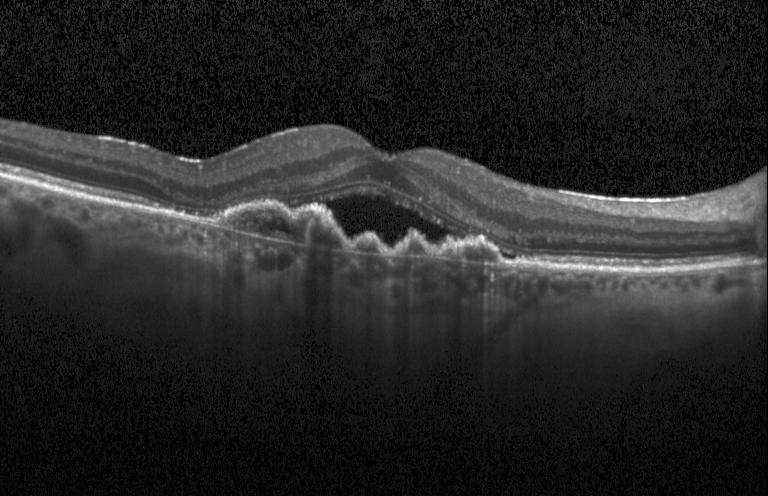

OCT B-scan. Diagnosis: a choroidal neovascular membrane.